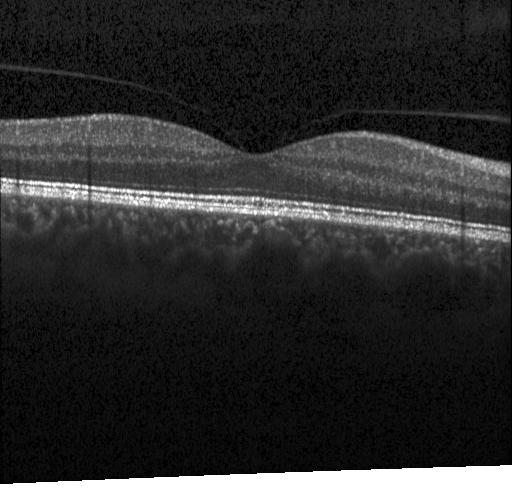

Finding: neither CNV, DME, nor drusen.